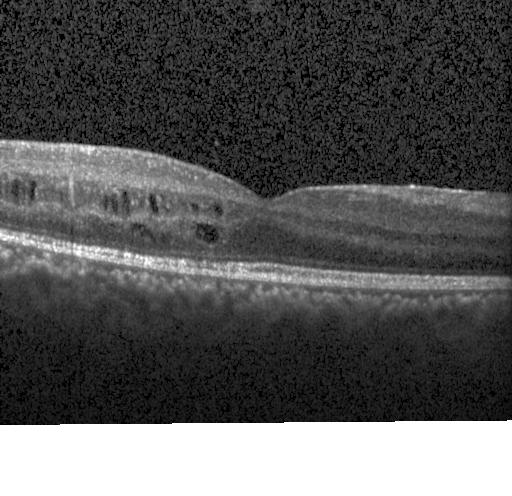 OCT B-scan; centered on the fovea; spectral-domain optical coherence tomography; Heidelberg Spectralis OCT system.
The scan shows diabetic macular edema (DME).